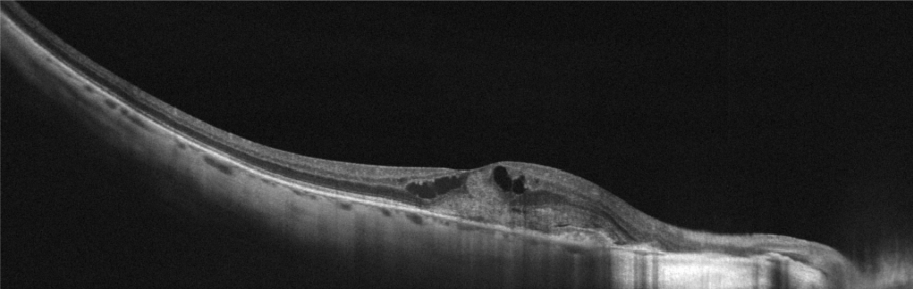
OCT B-scan. Through the macula. Optovue Avanti RTVue XR — Finding: age-related macular degeneration.